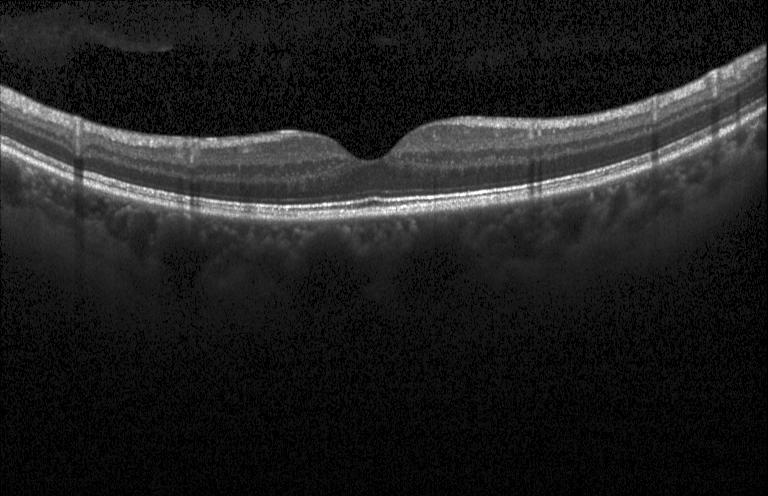

Centered on the fovea; retinal OCT cross-section; spectral-domain optical coherence tomography
Neither choroidal neovascularization, diabetic macular edema, nor drusen.